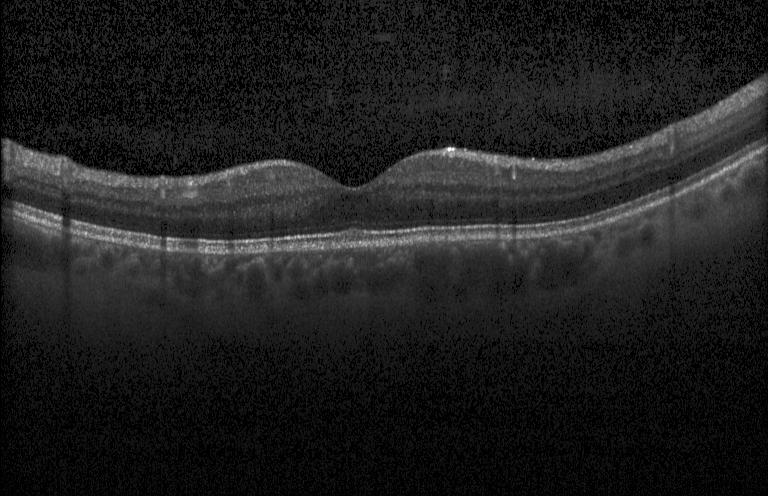

Centered on the fovea · Heidelberg Spectralis · spectral-domain optical coherence tomography · retinal OCT B-scan
Assessment: no choroidal neovascularization, diabetic macular edema, or drusen.